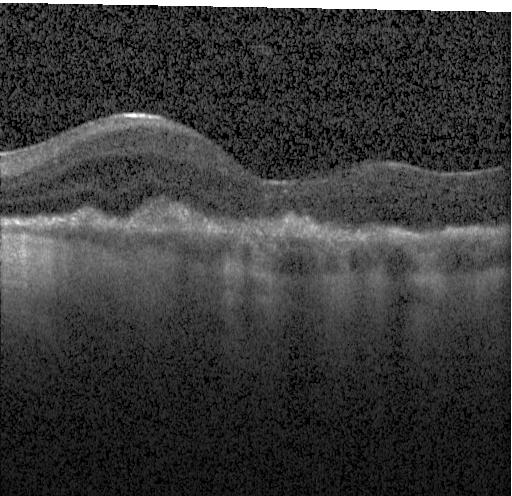 OCT scan showing choroidal neovascularization (CNV).